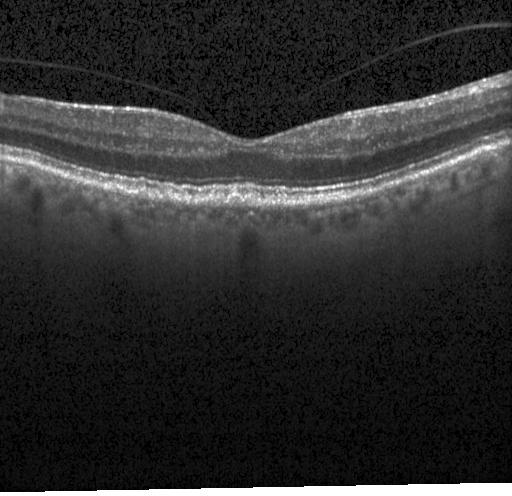 Multiple drusen.